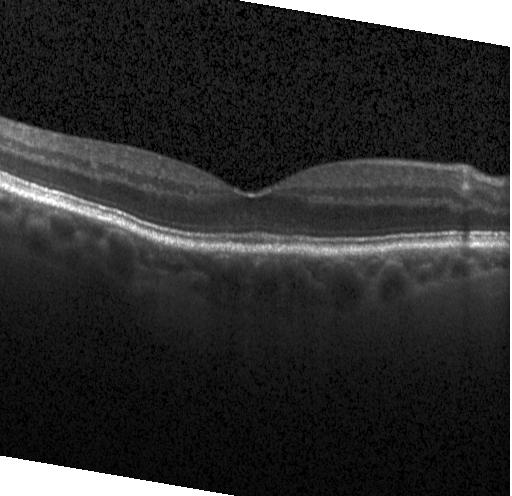

Optical coherence tomography scan
Impression: neither CNV, DME, nor drusen.